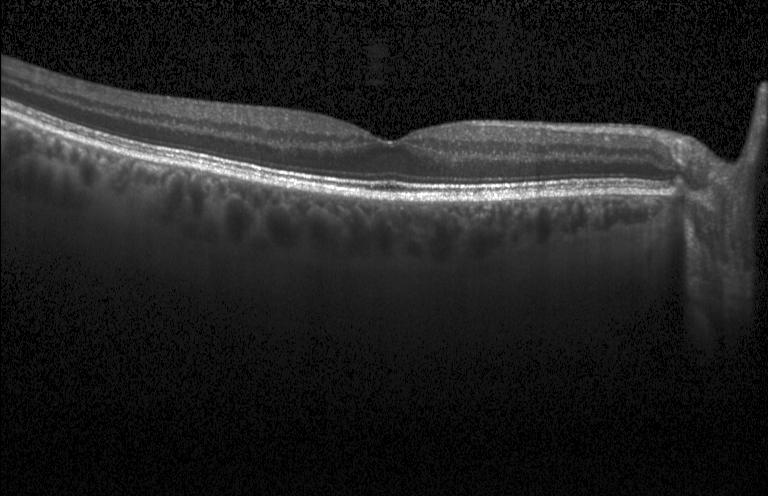
Optical coherence tomography scan — Assessment: no evidence of CNV, DME, or drusen.